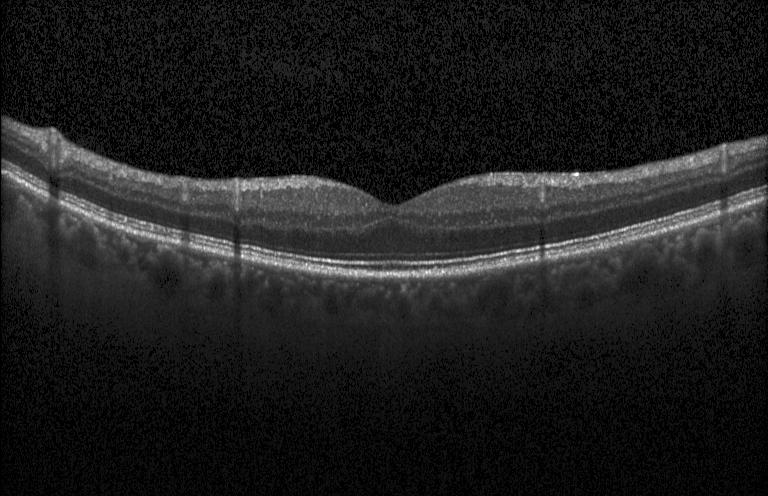 Centered on the fovea · retinal OCT B-scan · instrument: Heidelberg Spectralis · spectral-domain OCT — Impression: no evidence of CNV, DME, or drusen.